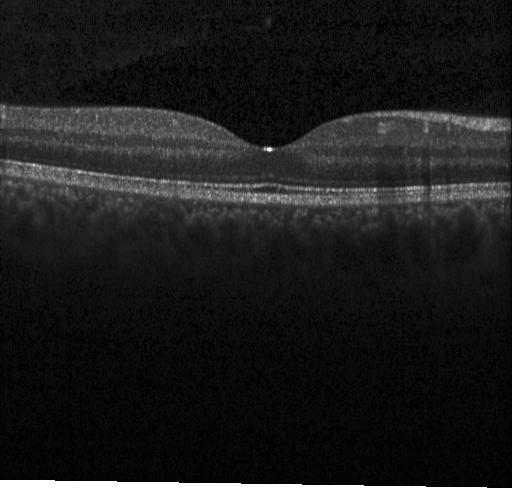 Diagnosis: neither CNV, DME, nor drusen.